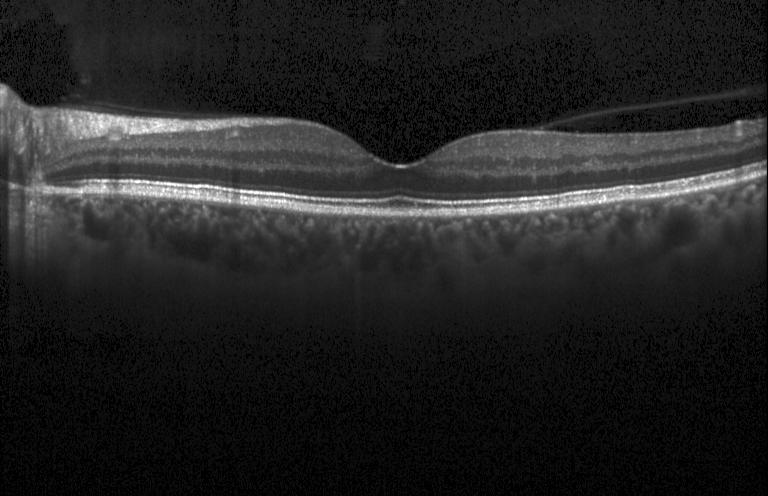
Macular OCT: no evidence of CNV, DME, or drusen.